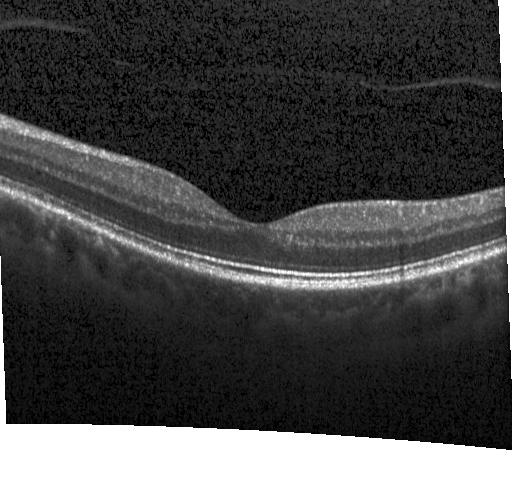 SD-OCT. OCT line scan.
Finding: neither choroidal neovascularization, diabetic macular edema, nor drusen.